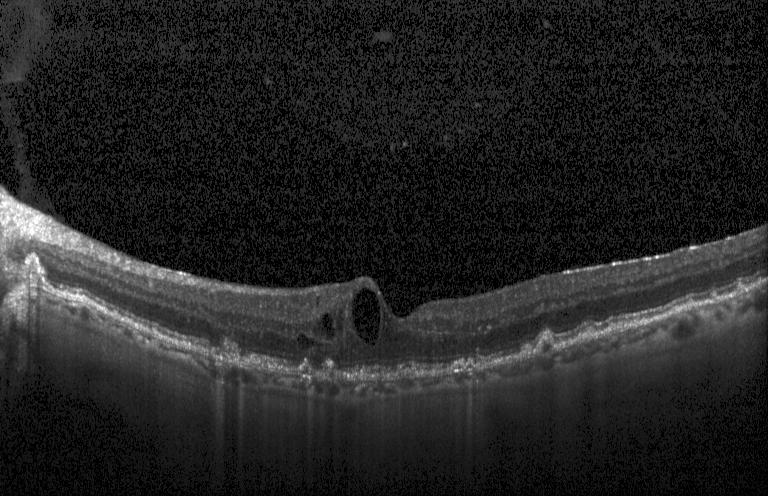
Finding: choroidal neovascularization.